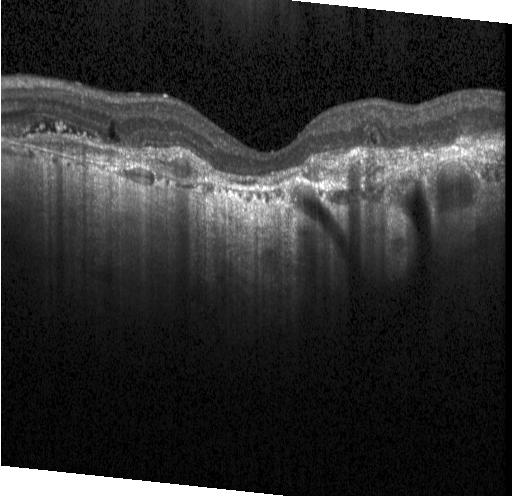 Impression: a choroidal neovascular membrane.